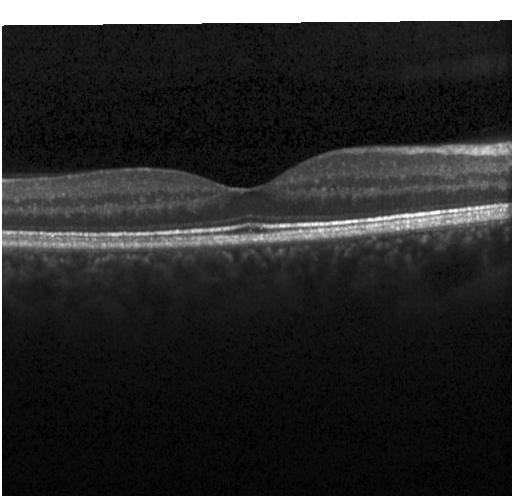

OCT line scan, centered on the fovea, Heidelberg Spectralis OCT system.
Assessment: no choroidal neovascularization, diabetic macular edema, or drusen.